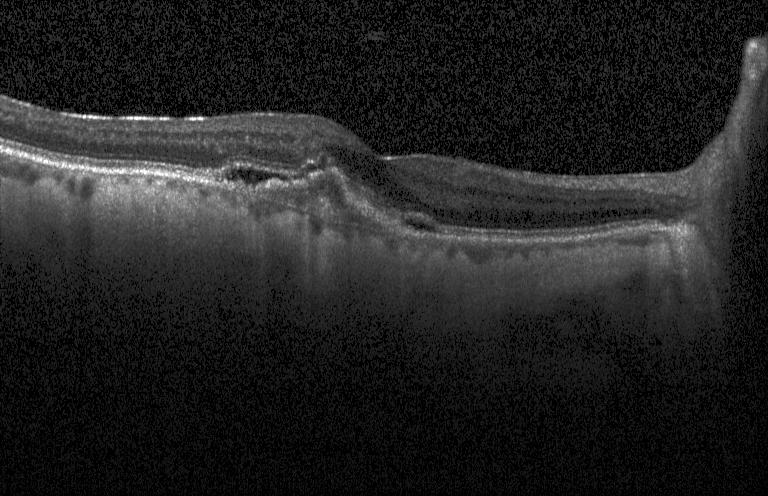

The scan shows choroidal neovascularization.